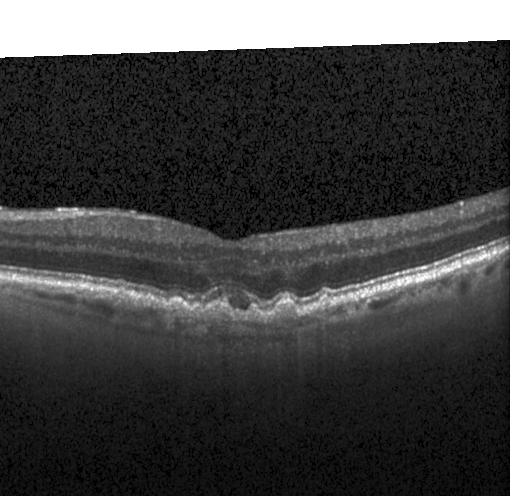

Retinal OCT cross-section. Acquired on a Heidelberg Spectralis — Diagnosis: choroidal neovascularization.